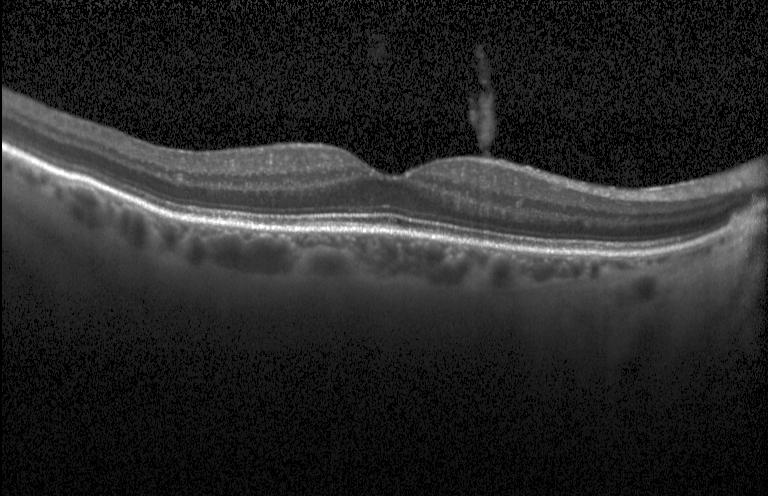 Optical coherence tomography B-scan
Impression: no choroidal neovascularization, diabetic macular edema, or drusen.